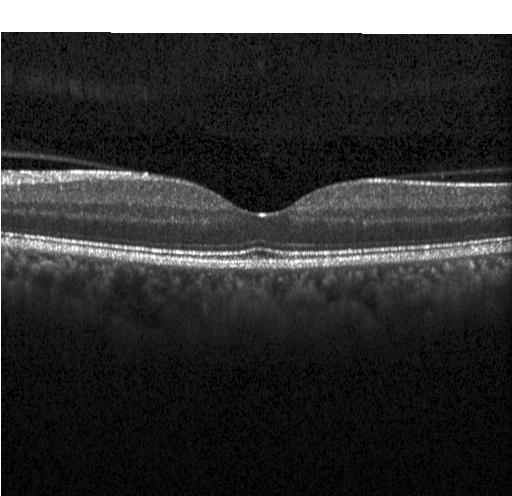

Horizontal scan through the fovea; optical coherence tomography B-scan — Macular OCT: no choroidal neovascularization, no diabetic macular edema, and no drusen.